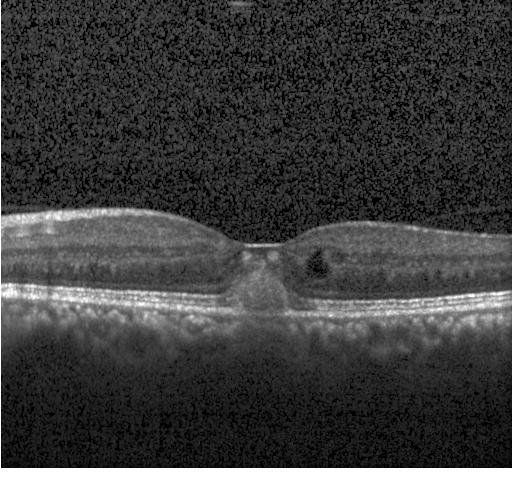

Heidelberg Spectralis OCT system · retinal OCT cross-section · centered on the fovea · spectral-domain optical coherence tomography. Assessment: choroidal neovascularization.